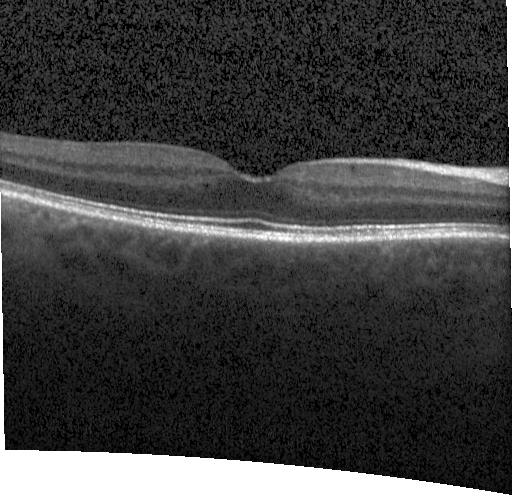 Assessment: no evidence of choroidal neovascularization, diabetic macular edema, or drusen.